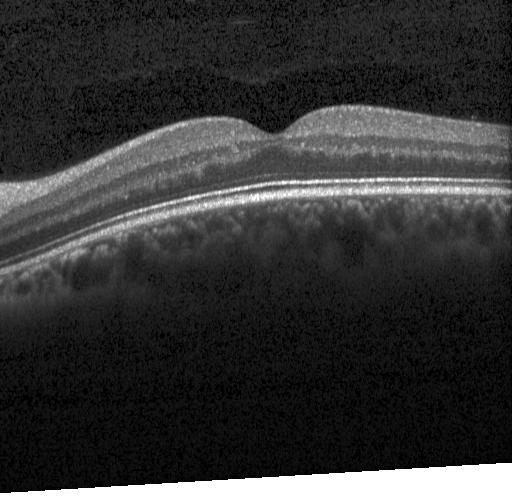 Retinal OCT cross-section. Through the macula
OCT finding: no evidence of choroidal neovascularization, diabetic macular edema, or drusen.